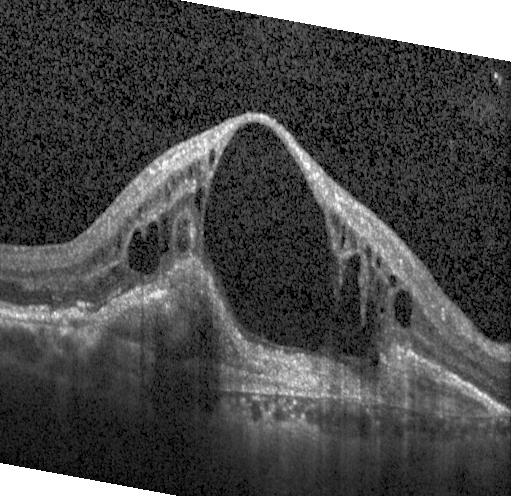
OCT line scan · fovea-centered — Finding: choroidal neovascularization.